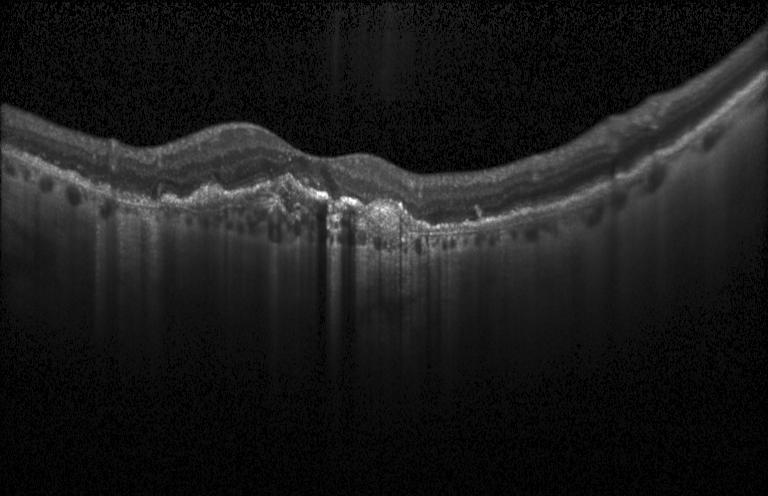
Macular OCT: a choroidal neovascular membrane.